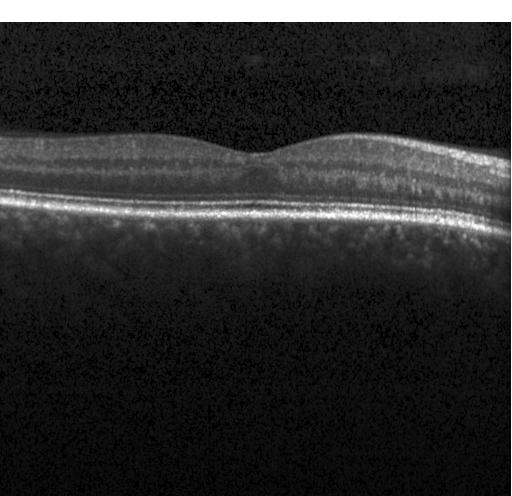
Acquired on a Heidelberg Spectralis · macular scan · optical coherence tomography scan · SD-OCT.
Finding: no evidence of choroidal neovascularization, diabetic macular edema, or drusen.